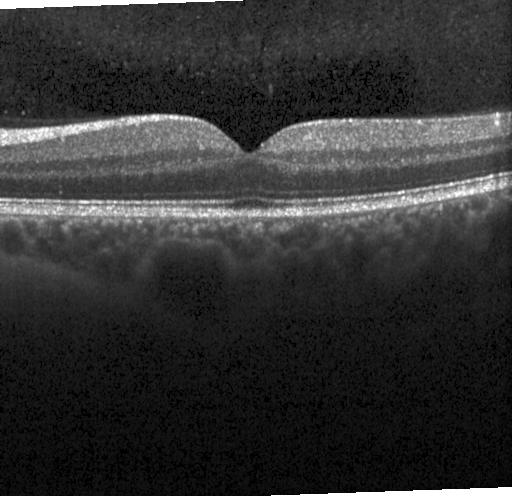

Spectral-domain optical coherence tomography · OCT B-scan · instrument: Heidelberg Spectralis · horizontal scan through the fovea
Finding: neither choroidal neovascularization, diabetic macular edema, nor drusen.